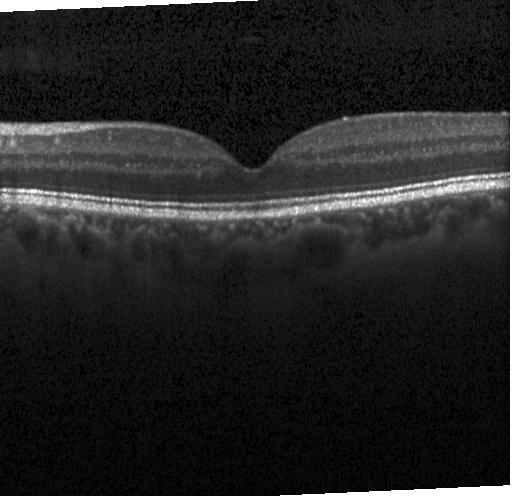

Spectral-domain OCT; optical coherence tomography B-scan — Diagnosis: no CNV, no DME, and no drusen.